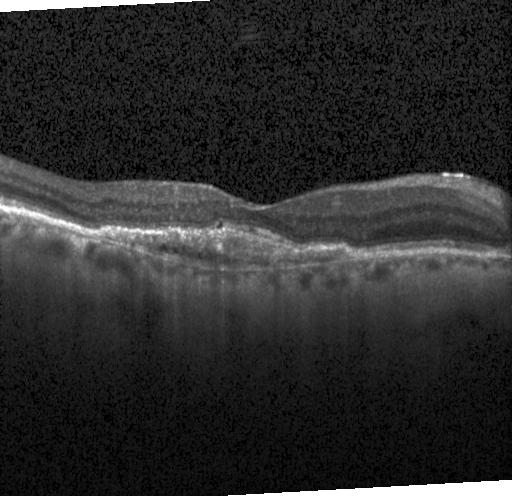 Retinal OCT cross-section showing a choroidal neovascular membrane.